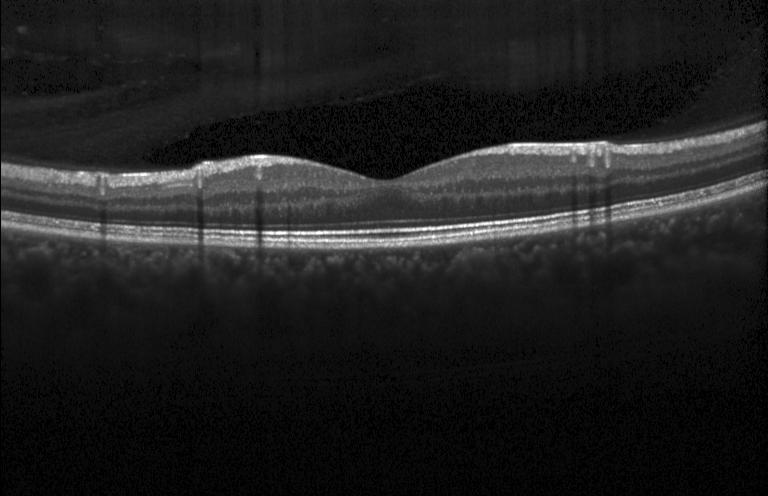 This B-scan demonstrates neither choroidal neovascularization, diabetic macular edema, nor drusen.